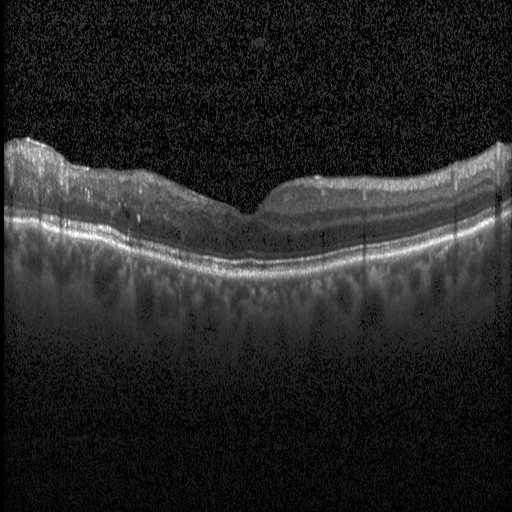 Retinal OCT B-scan
This B-scan demonstrates DME.